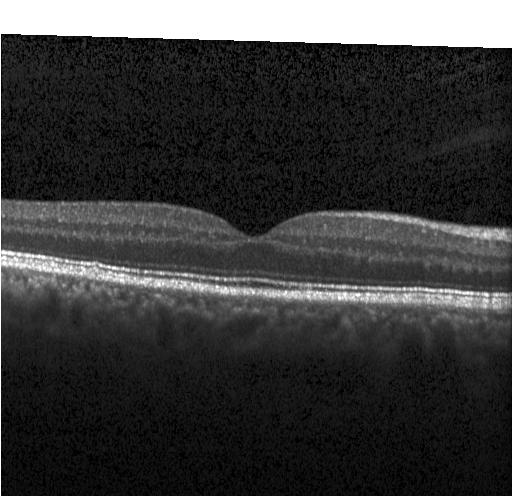

Diagnosis: no choroidal neovascularization, no diabetic macular edema, and no drusen.